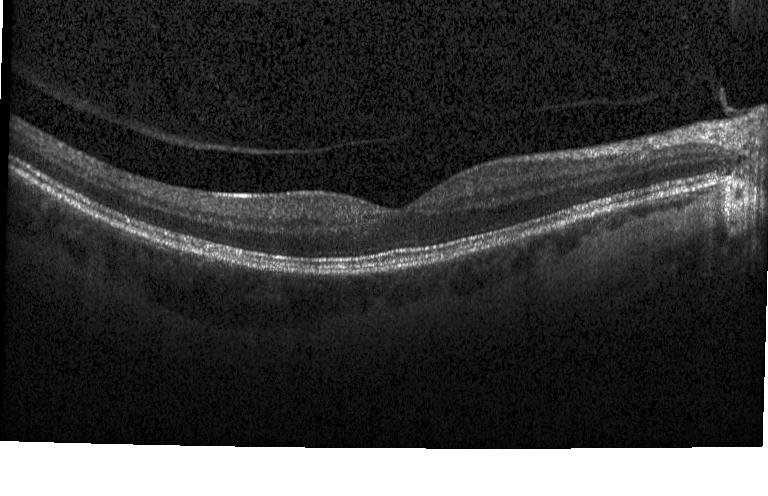
Retinal OCT cross-section. The scan shows no evidence of choroidal neovascularization, diabetic macular edema, or drusen.